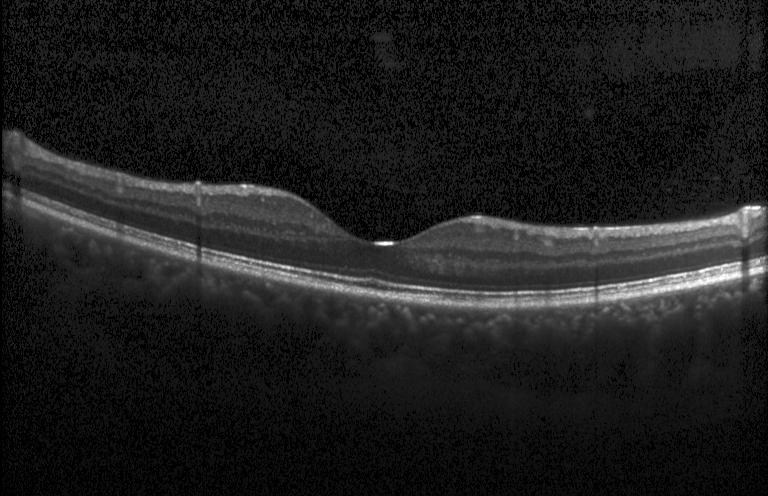

Heidelberg Spectralis, horizontal scan through the fovea, optical coherence tomography B-scan, spectral-domain optical coherence tomography
Impression: no CNV, DME, or drusen.